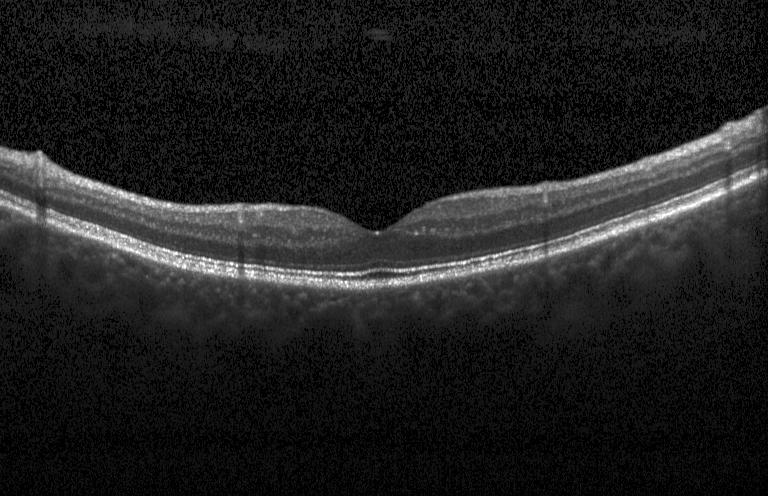
Dx: no evidence of choroidal neovascularization, diabetic macular edema, or drusen.